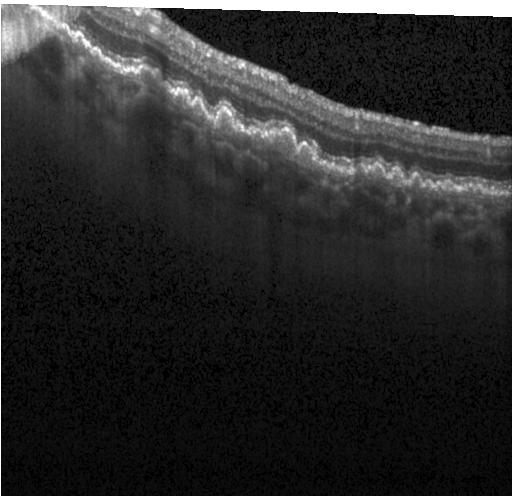 Finding: CNV.